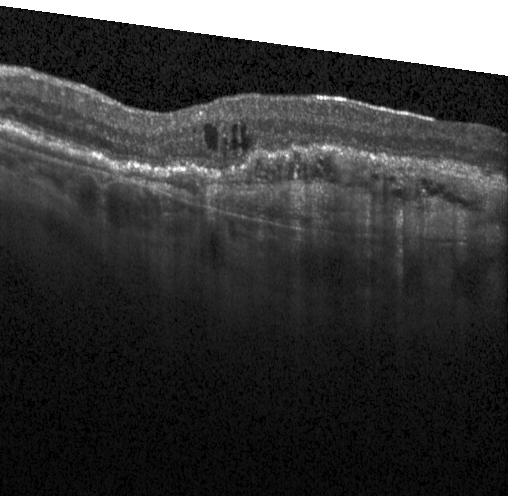 Instrument: Heidelberg Spectralis. Spectral-domain OCT. Centered on the fovea. Retinal OCT B-scan. Choroidal neovascularization (CNV).